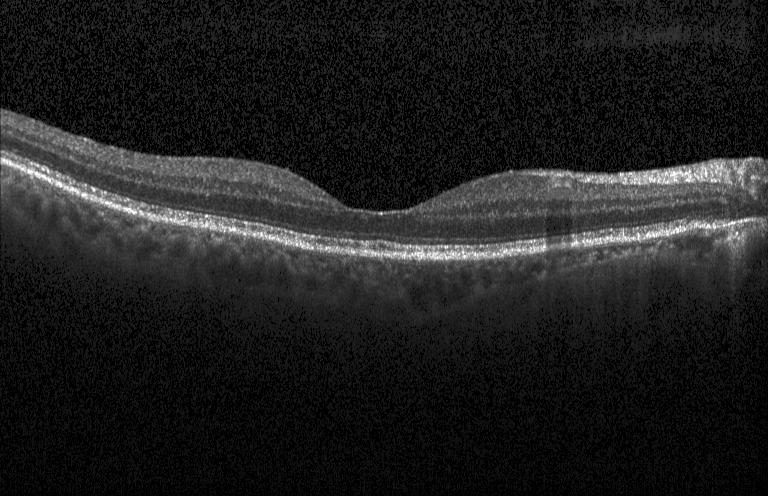 Diagnosis: no evidence of CNV, DME, or drusen.